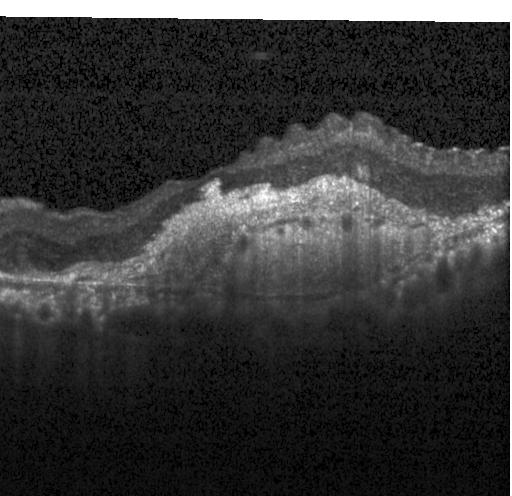

Heidelberg Spectralis OCT system. OCT B-scan — Assessment: a choroidal neovascular membrane.